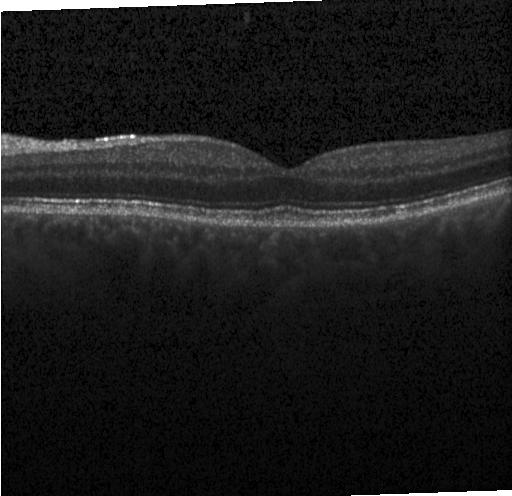

OCT line scan, Heidelberg Spectralis
Impression: no choroidal neovascularization, diabetic macular edema, or drusen.